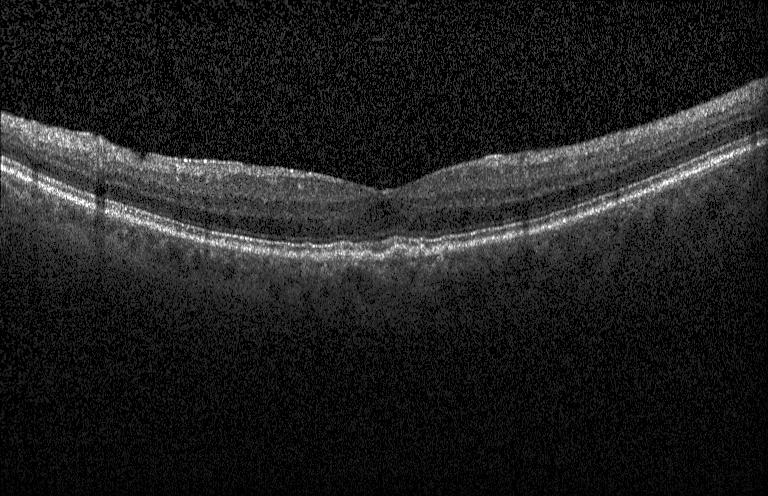

Spectral-domain optical coherence tomography, optical coherence tomography scan. The scan shows multiple drusen.